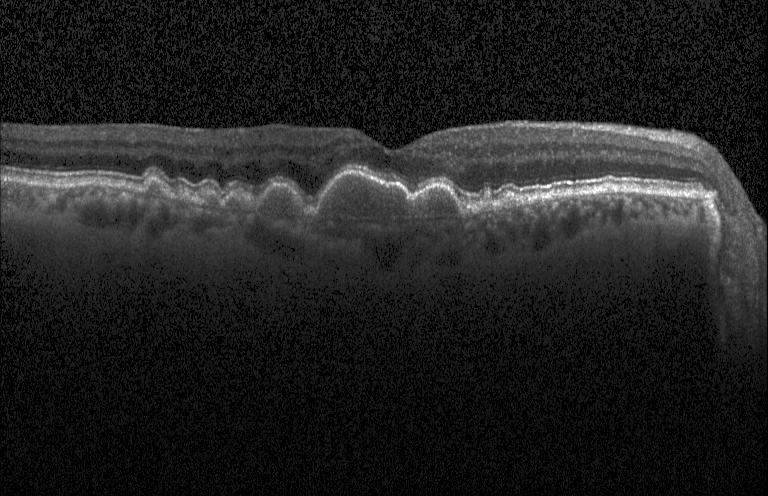

SD-OCT, OCT B-scan, acquired on a Heidelberg Spectralis, macular scan. OCT finding: sub-RPE drusenoid deposits.